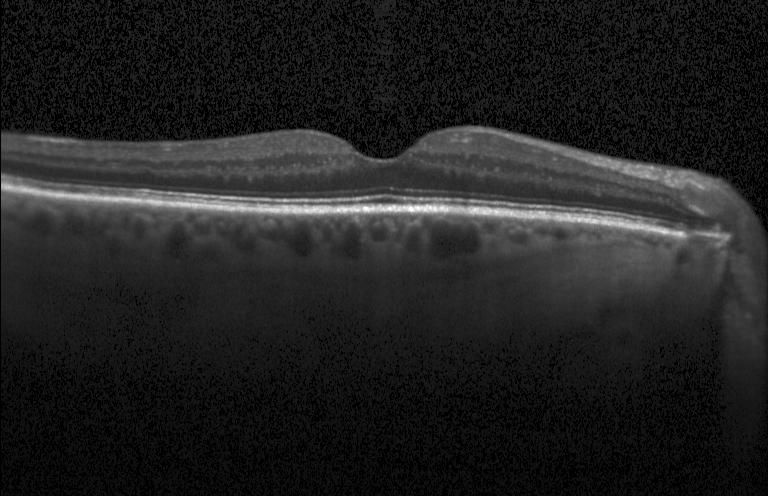 Assessment: no choroidal neovascularization, no diabetic macular edema, and no drusen.